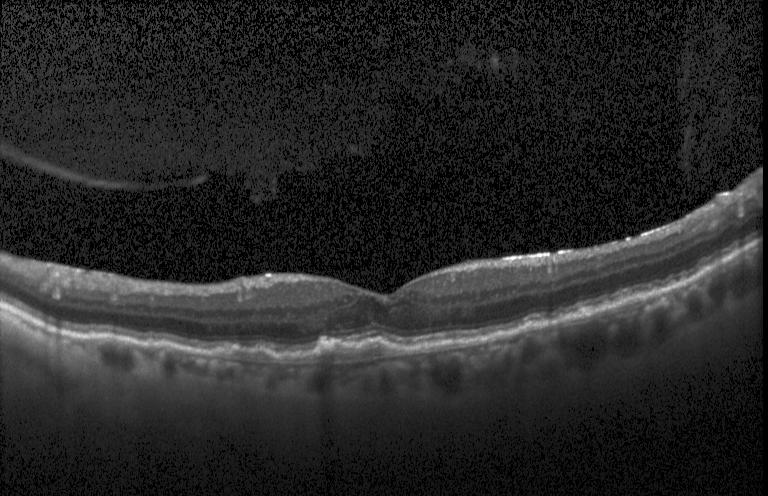 This B-scan demonstrates CNV.